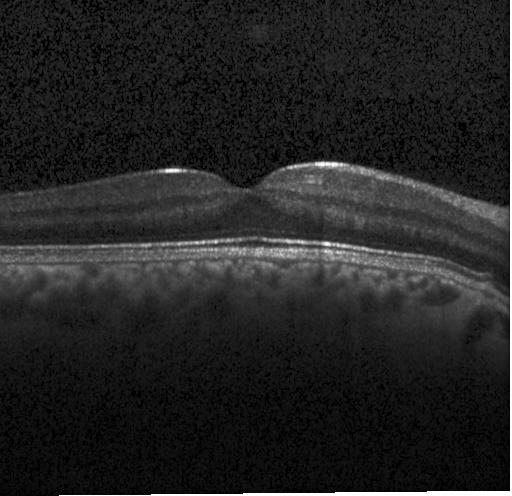

Horizontal scan through the fovea · Heidelberg Spectralis OCT system · spectral-domain optical coherence tomography · OCT line scan
No evidence of choroidal neovascularization, diabetic macular edema, or drusen.